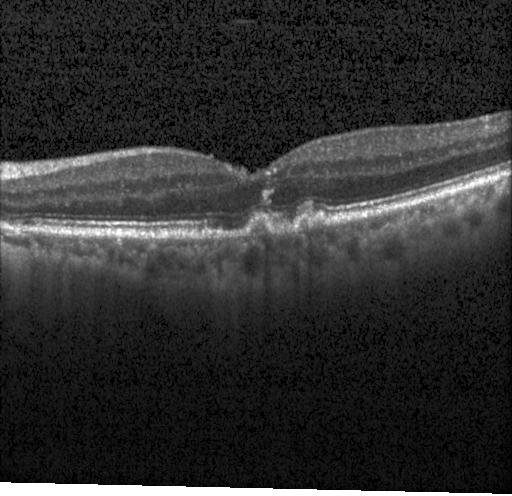

OCT line scan.
Dx: multiple drusen.